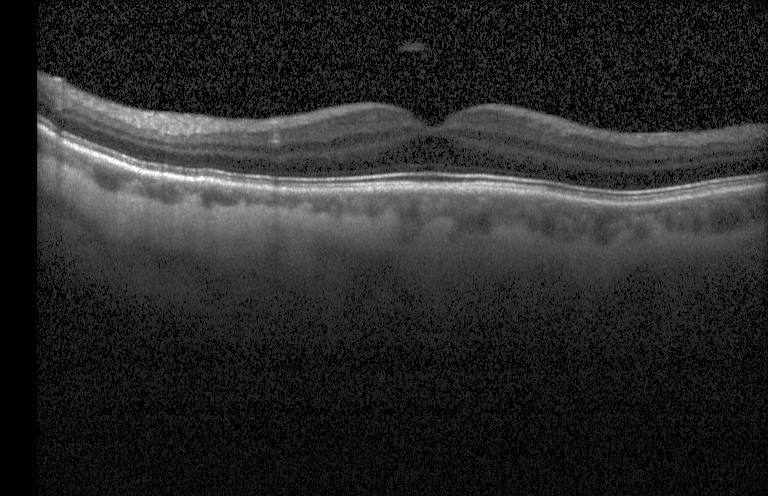

The scan shows no choroidal neovascularization, diabetic macular edema, or drusen.